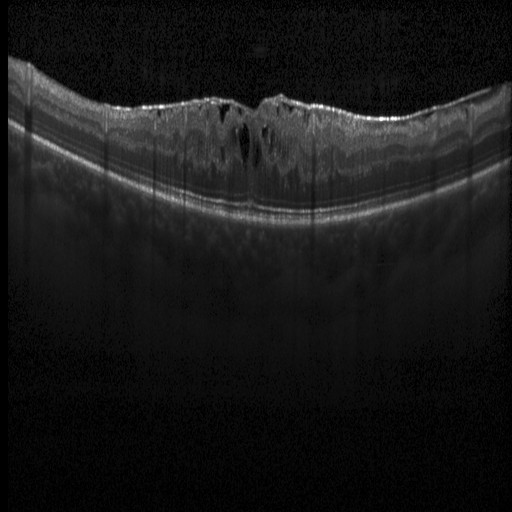

Retinal OCT cross-section, instrument: Heidelberg Spectralis, spectral-domain optical coherence tomography, centered on the fovea
Assessment: diabetic macular edema (DME).